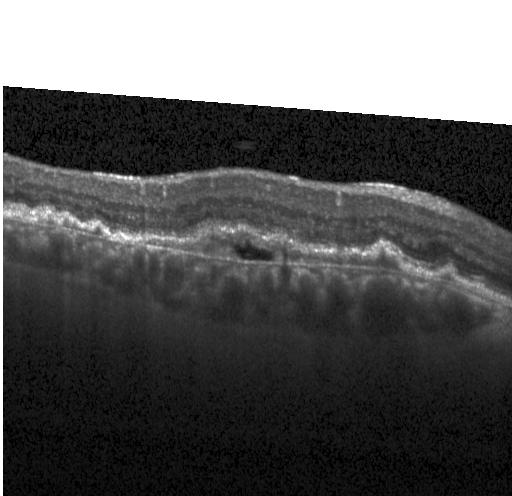

Spectral-domain OCT, Heidelberg Spectralis OCT system, OCT line scan
Dx: a choroidal neovascular membrane.